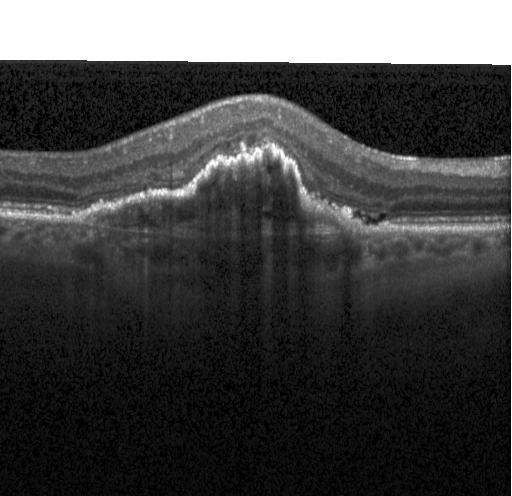

Macular scan. Heidelberg Spectralis OCT system. OCT line scan. Spectral-domain OCT — A choroidal neovascular membrane.